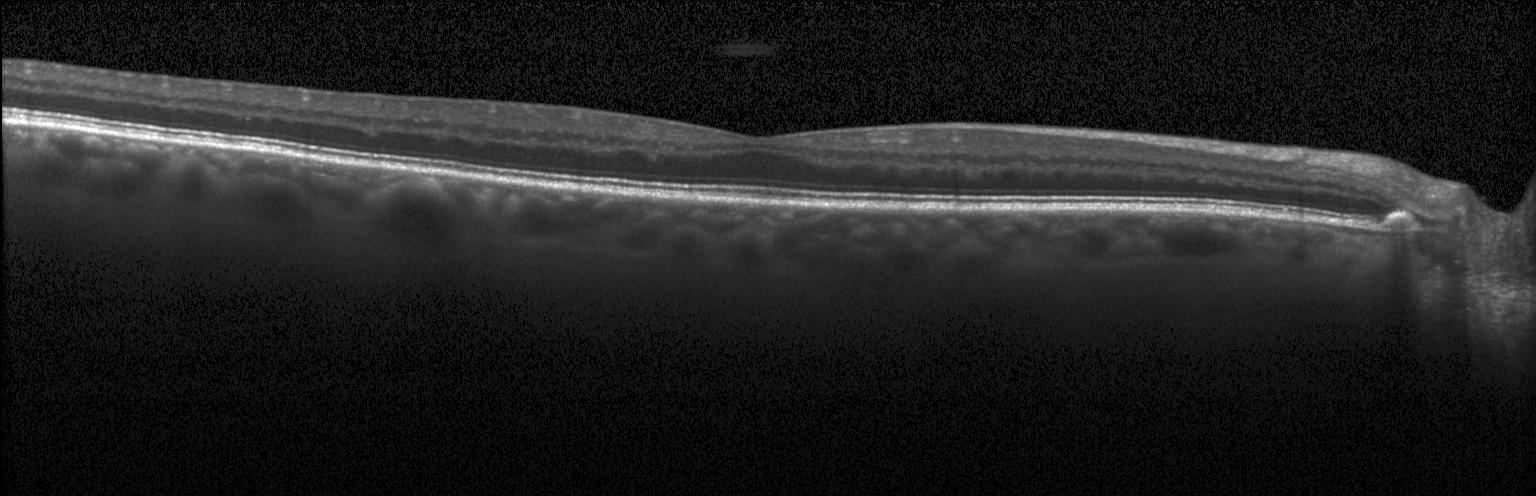

Heidelberg Spectralis, through the macula, spectral-domain optical coherence tomography, OCT B-scan.
Macular OCT: no CNV, DME, or drusen.